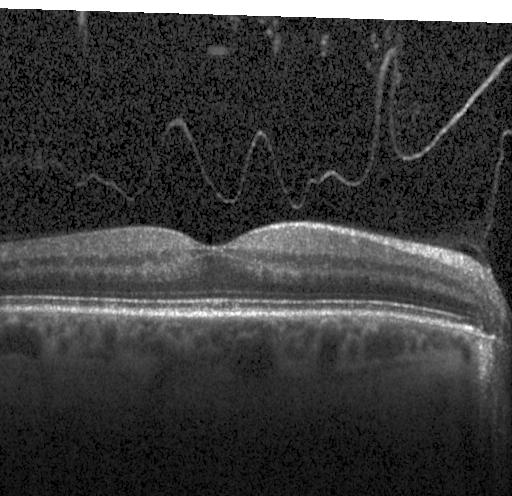

Impression: no choroidal neovascularization, diabetic macular edema, or drusen.